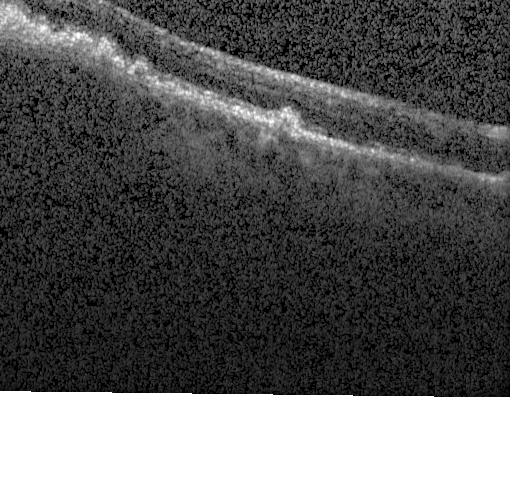
OCT finding: drusen.